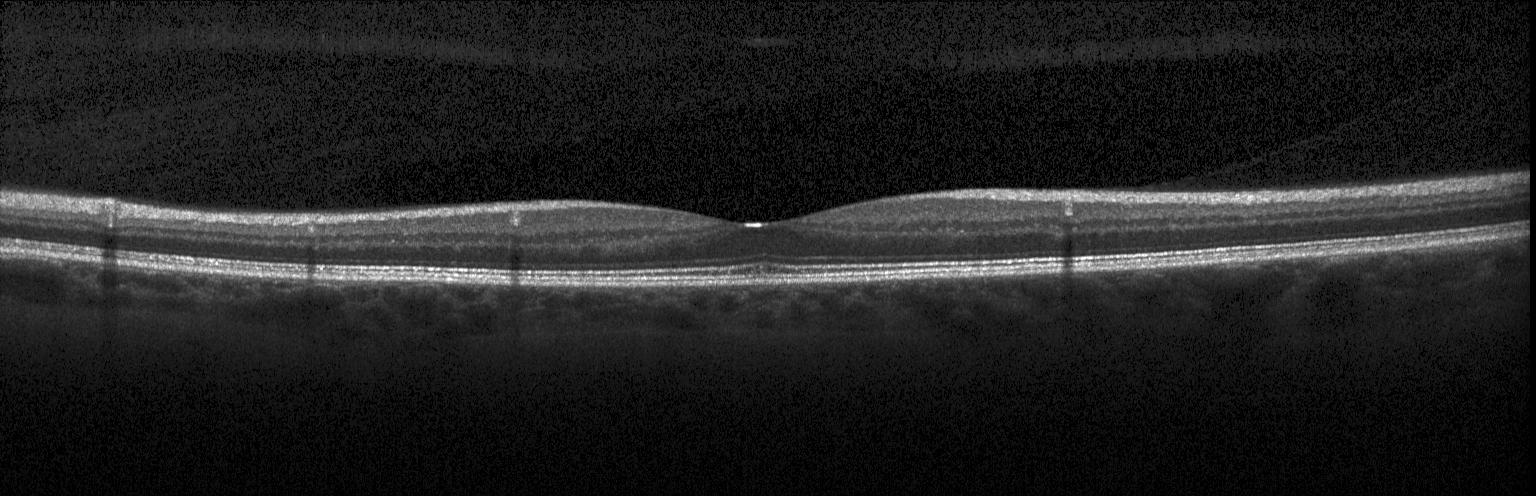
Macular scan · acquired on a Heidelberg Spectralis · spectral-domain optical coherence tomography · retinal OCT cross-section
OCT finding: no CNV, no DME, and no drusen.